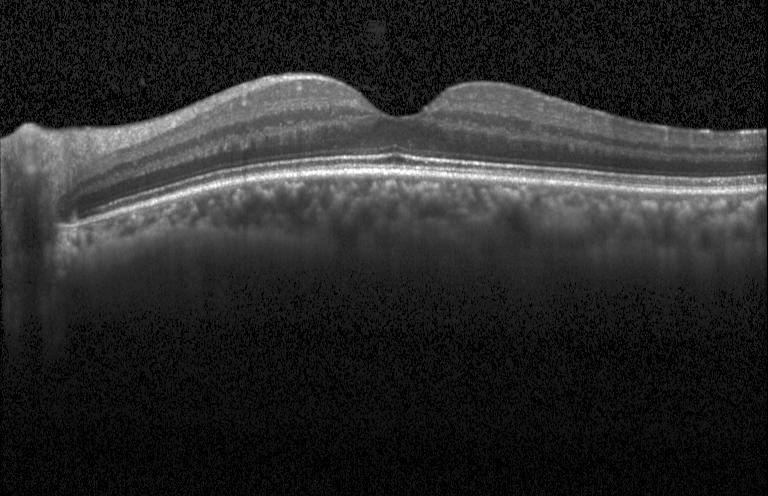
This B-scan demonstrates neither choroidal neovascularization, diabetic macular edema, nor drusen.